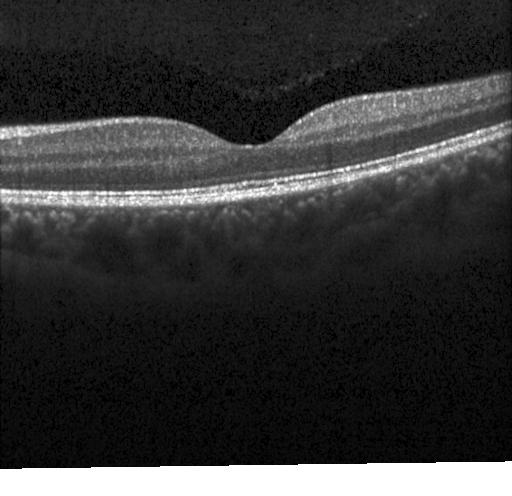

Optical coherence tomography B-scan.
OCT finding: no CNV, DME, or drusen.